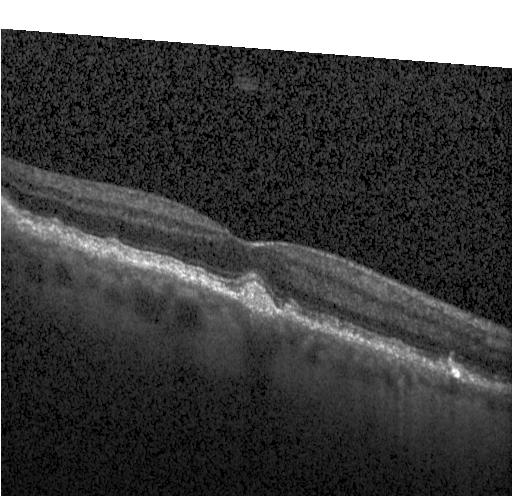 Horizontal scan through the fovea · OCT B-scan. Finding: multiple drusen.